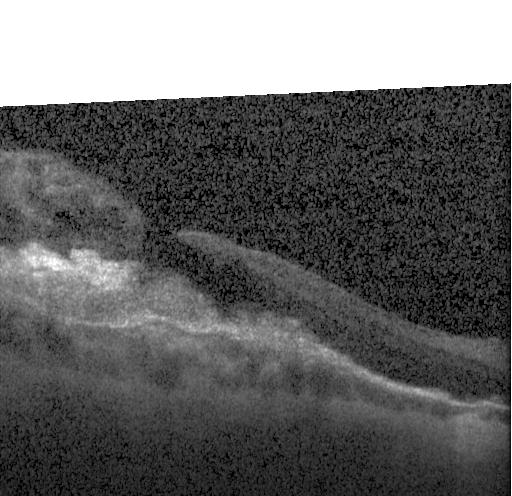
Centered on the fovea, retinal OCT cross-section
Dx: choroidal neovascularization (CNV).